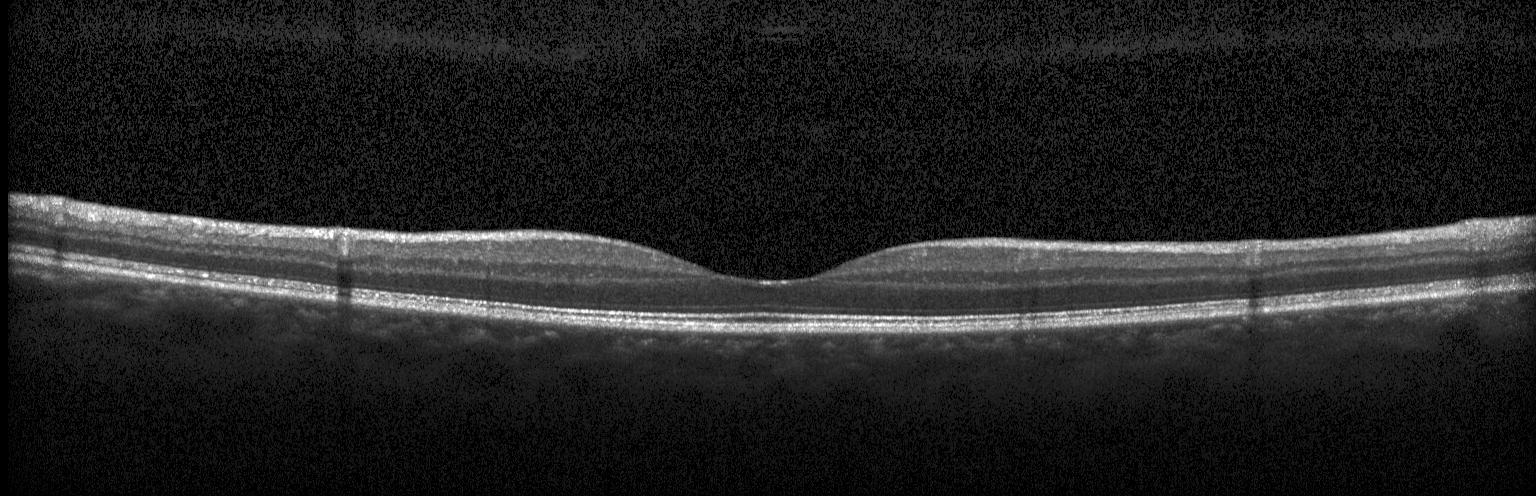
The scan shows no CNV, no DME, and no drusen.